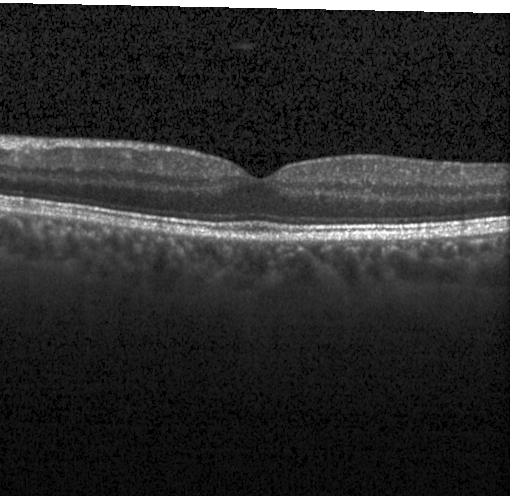

Impression: no choroidal neovascularization, no diabetic macular edema, and no drusen.